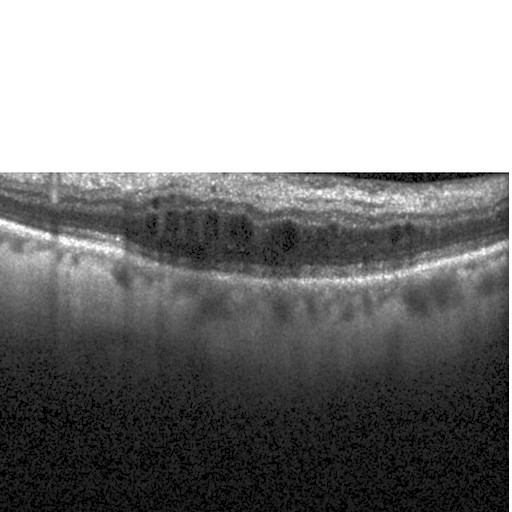 Macular OCT: diabetic macular edema.